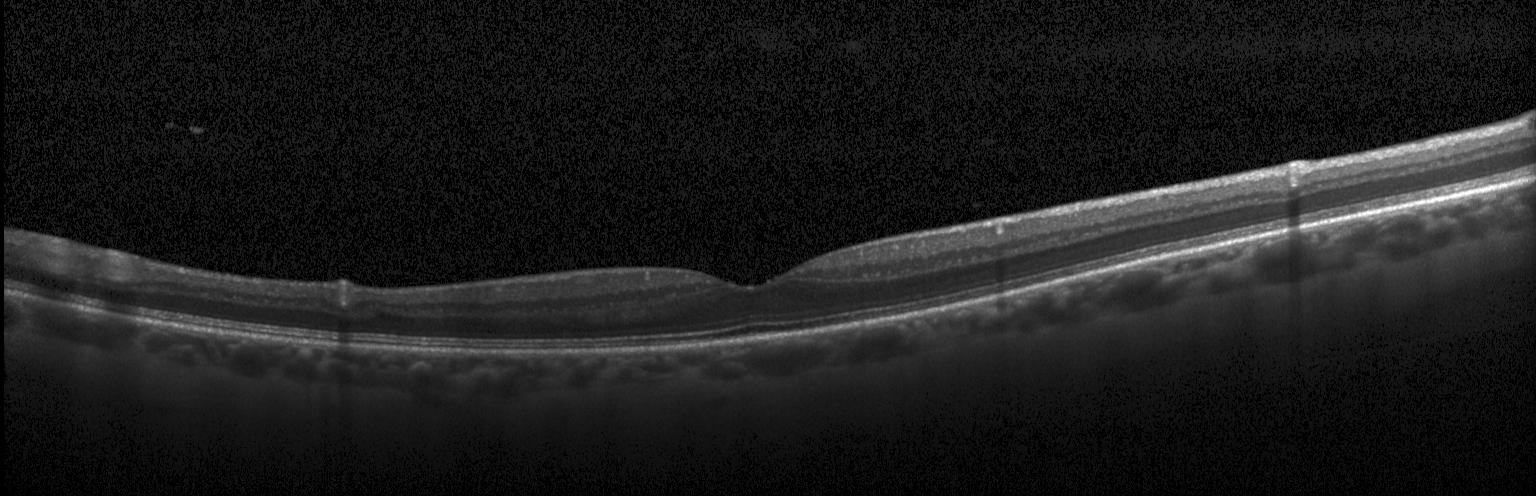
Optical coherence tomography B-scan · Heidelberg Spectralis · macular scan · spectral-domain optical coherence tomography.
No choroidal neovascularization, no diabetic macular edema, and no drusen.